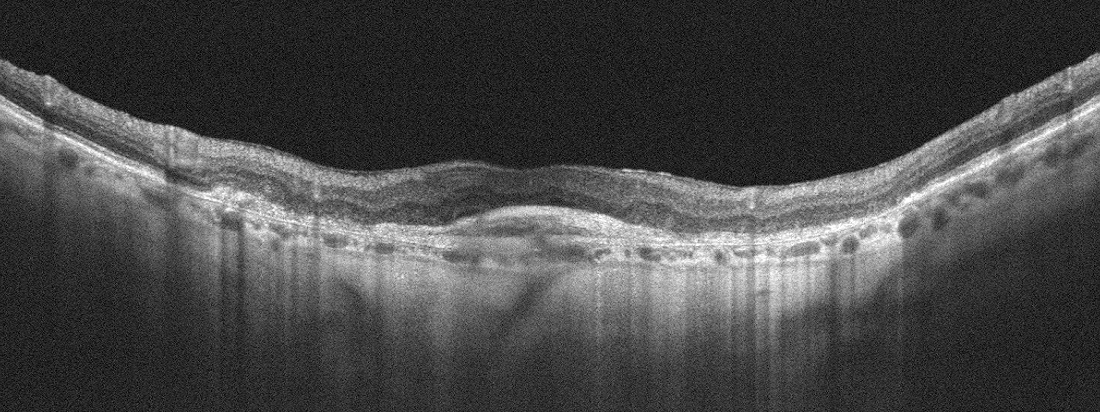

OCT line scan. Impression: age-related macular degeneration.